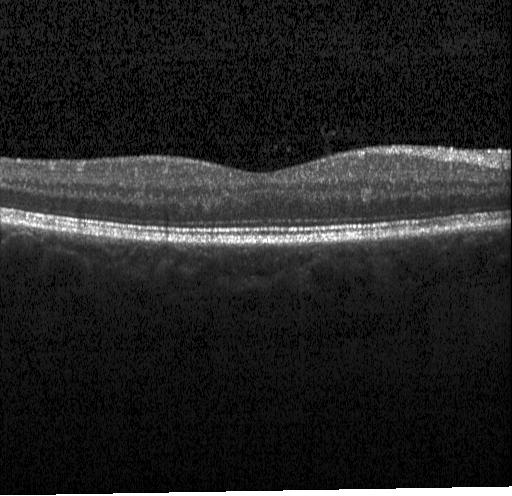
Optical coherence tomography scan — This B-scan demonstrates no CNV, no DME, and no drusen.